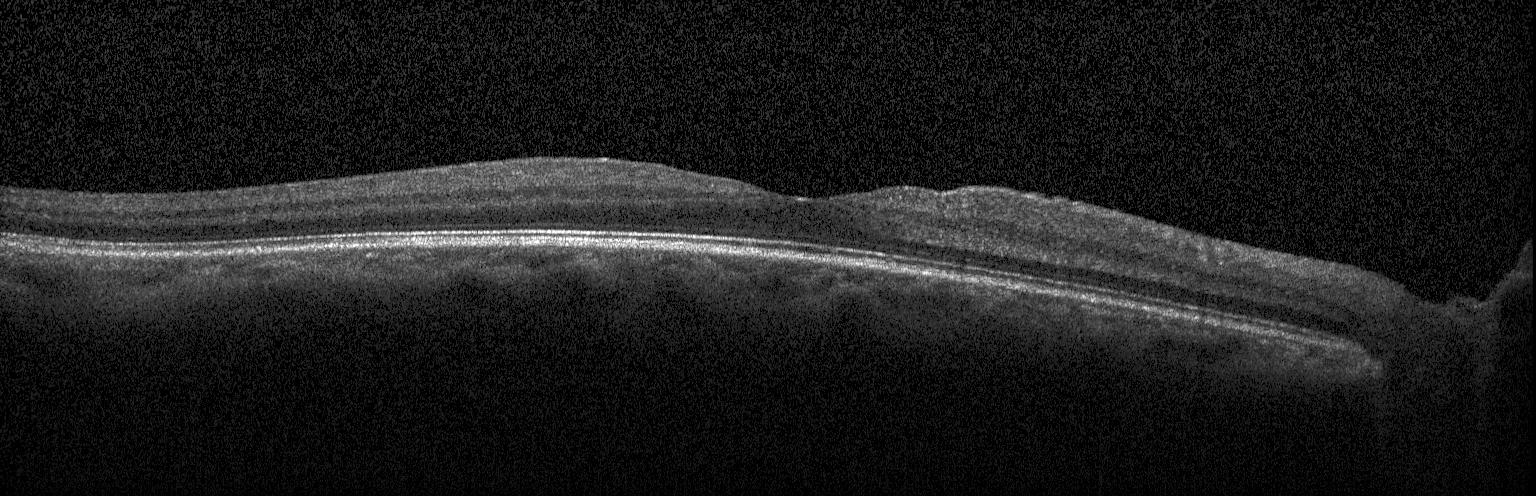 Optical coherence tomography B-scan.
Diagnosis: no choroidal neovascularization, no diabetic macular edema, and no drusen.